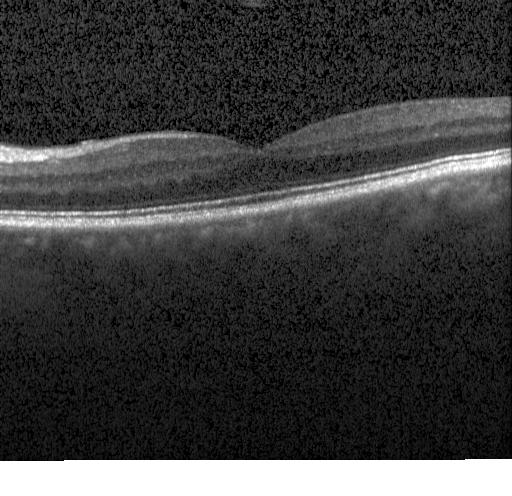
Finding: no evidence of choroidal neovascularization, diabetic macular edema, or drusen.